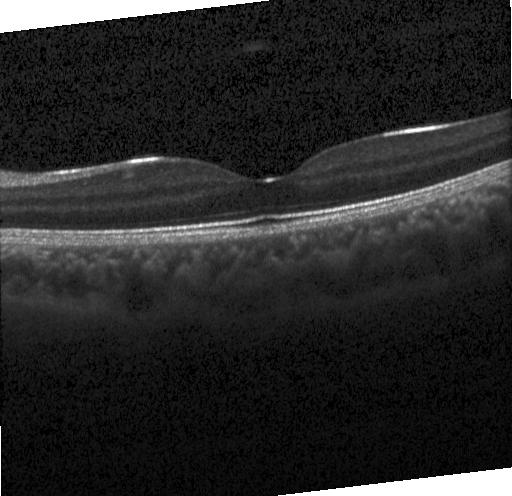 Finding: neither choroidal neovascularization, diabetic macular edema, nor drusen.